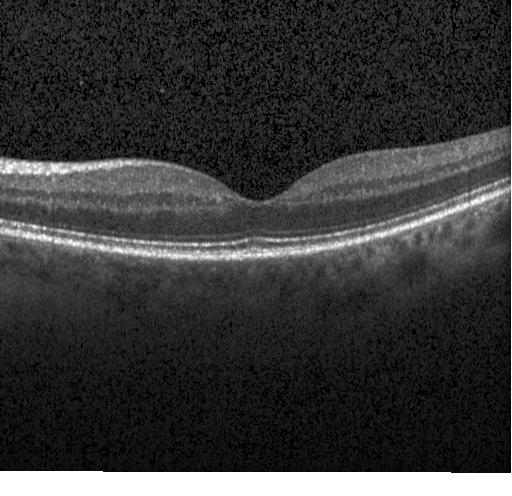
Diagnosis: neither CNV, DME, nor drusen.